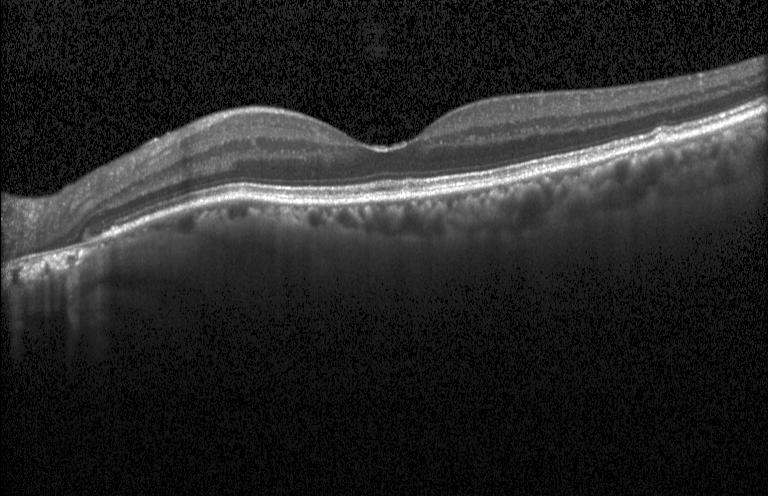

Finding: neither choroidal neovascularization, diabetic macular edema, nor drusen.